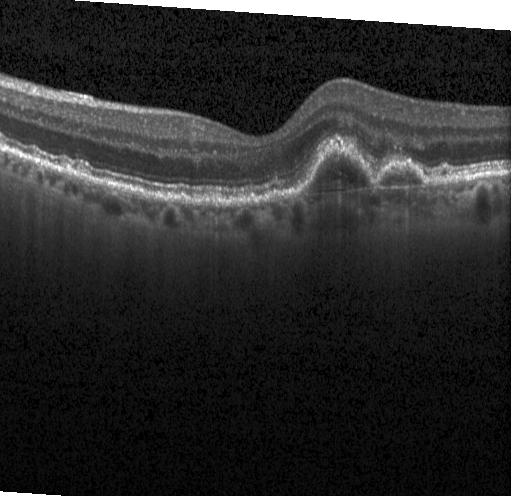 Instrument: Heidelberg Spectralis. Through the macula. SD-OCT. Optical coherence tomography scan. Dx: sub-RPE drusenoid deposits.